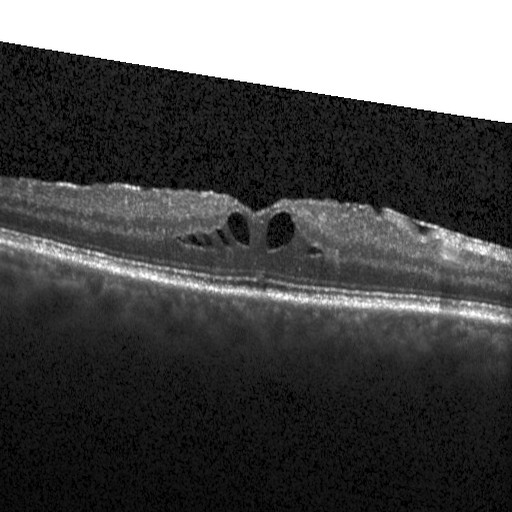 Macular OCT demonstrating diabetic macular edema.